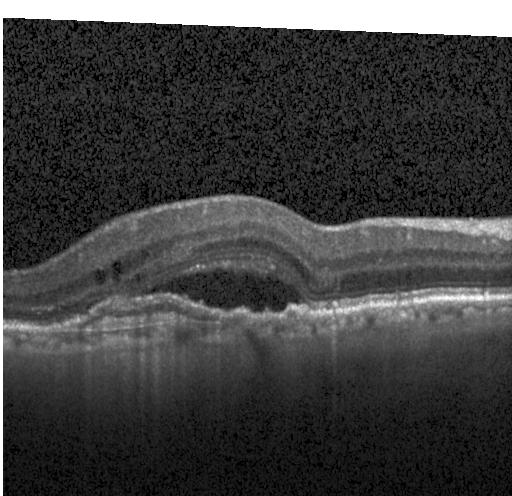

OCT B-scan. The scan shows choroidal neovascularization (CNV).